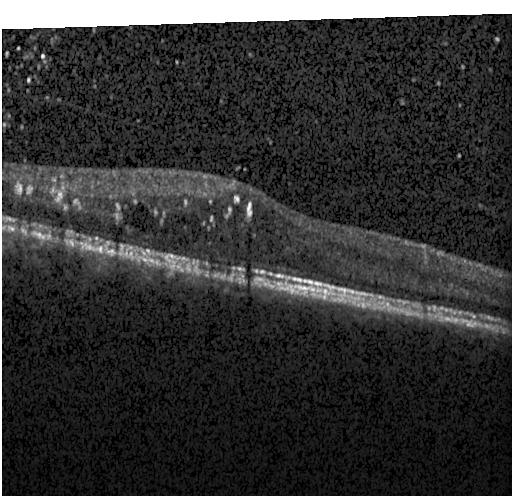 Spectral-domain OCT; optical coherence tomography B-scan
Finding: diabetic macular edema (DME).